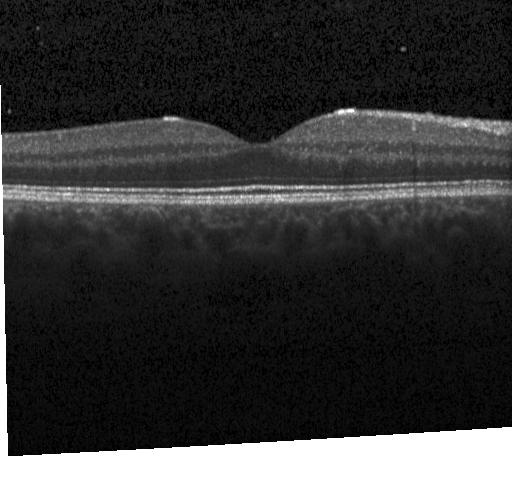

Heidelberg Spectralis OCT system, retinal OCT B-scan — Diagnosis: no evidence of CNV, DME, or drusen.